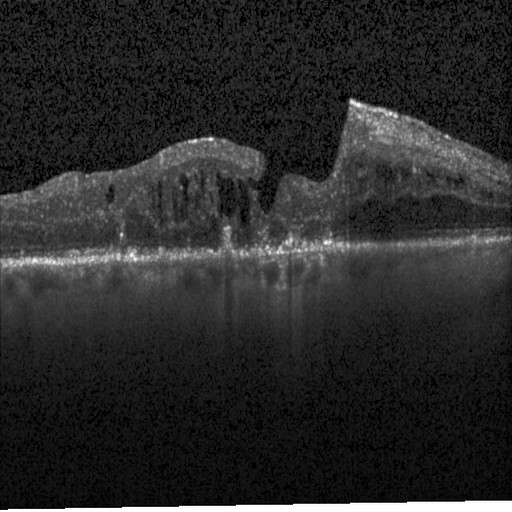
Instrument: Heidelberg Spectralis. Optical coherence tomography scan. Dx: diabetic macular edema (DME).